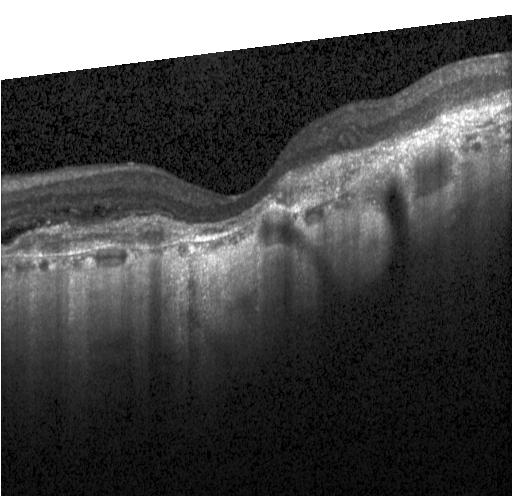 OCT B-scan showing choroidal neovascularization.